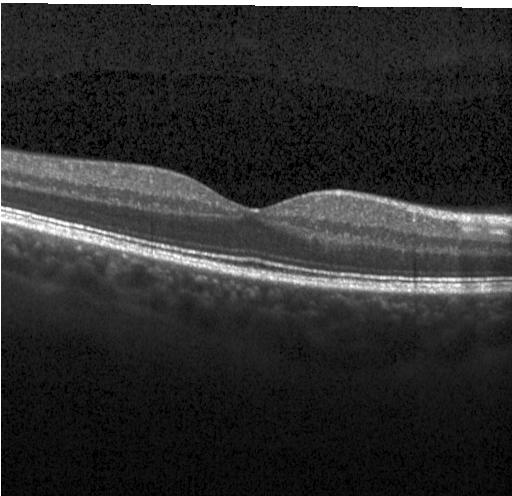 Retinal OCT B-scan. Heidelberg Spectralis OCT system. Through the macula. Spectral-domain OCT
Diagnosis: no choroidal neovascularization, diabetic macular edema, or drusen.